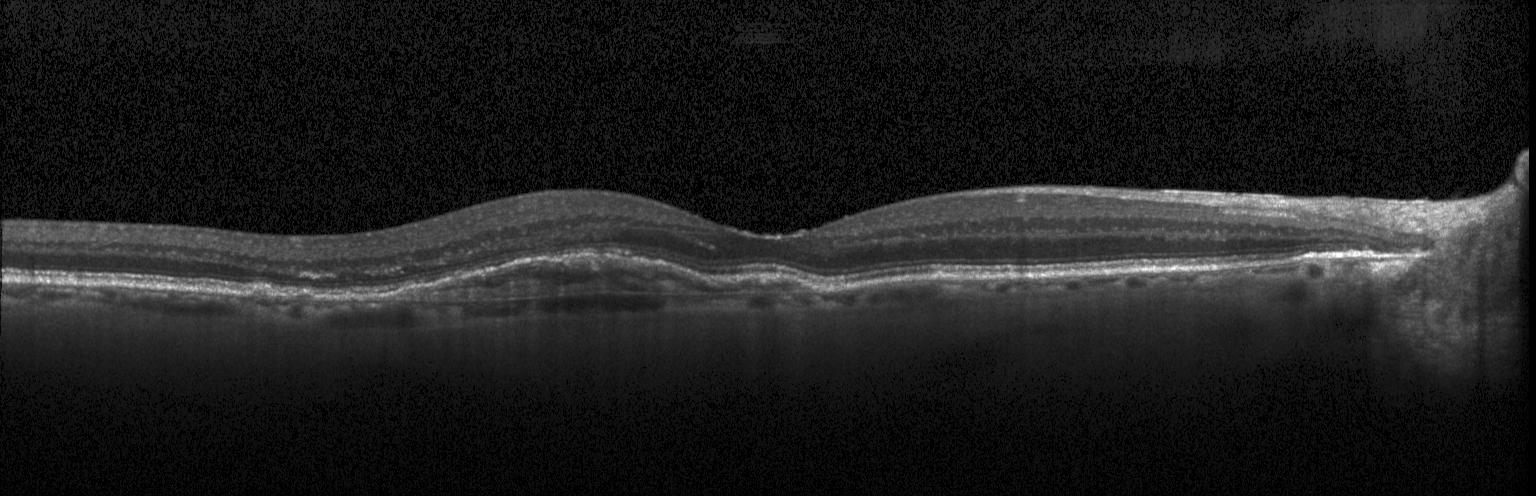 OCT B-scan.
Assessment: a choroidal neovascular membrane.